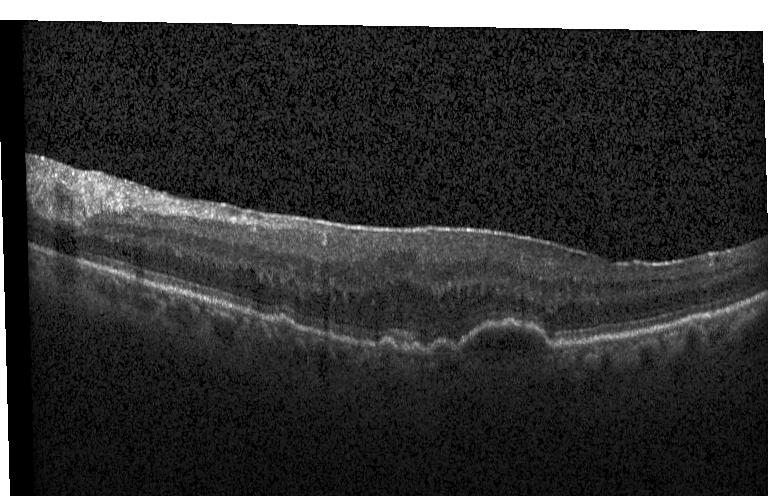 Macular OCT: a choroidal neovascular membrane.